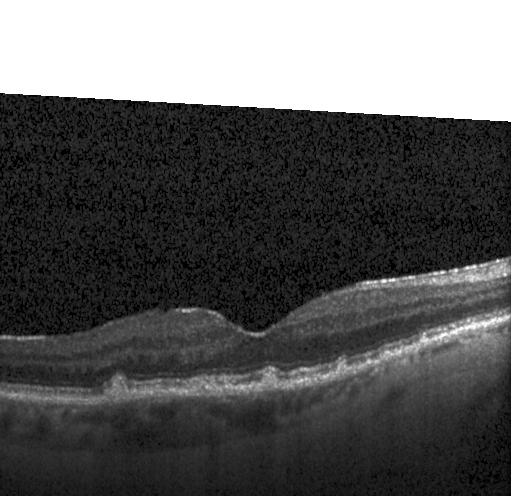

Fovea-centered. Optical coherence tomography B-scan. Instrument: Heidelberg Spectralis. Spectral-domain optical coherence tomography
Impression: drusen.